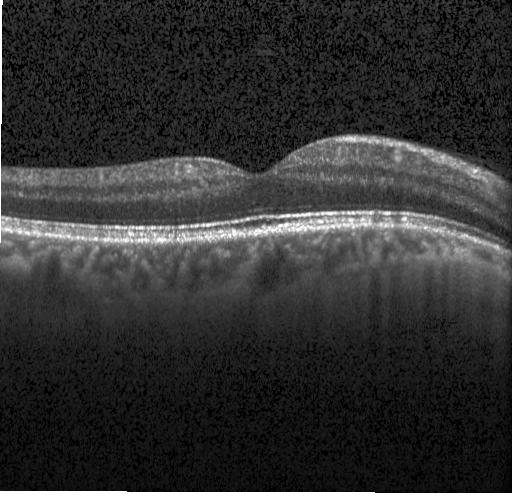
Finding: neither CNV, DME, nor drusen.